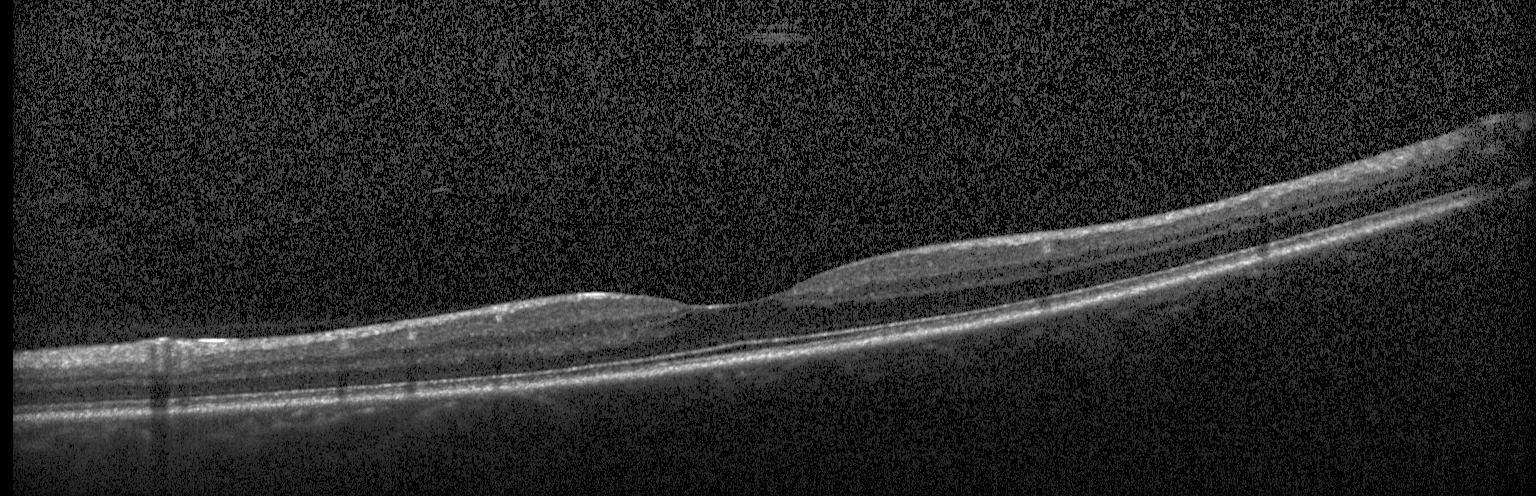
OCT line scan, through the macula, instrument: Heidelberg Spectralis, spectral-domain OCT
Diagnosis: no choroidal neovascularization, diabetic macular edema, or drusen.